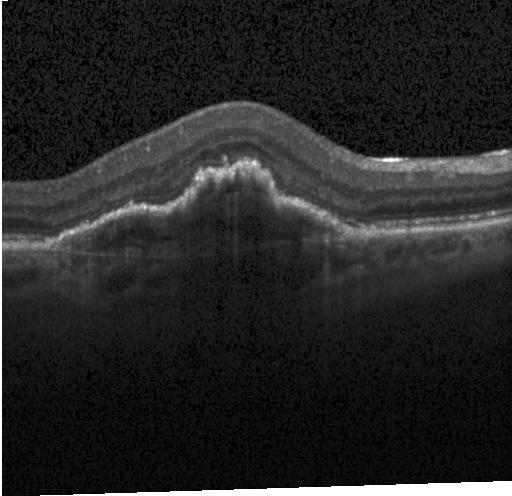
Optical coherence tomography B-scan. This B-scan demonstrates CNV.